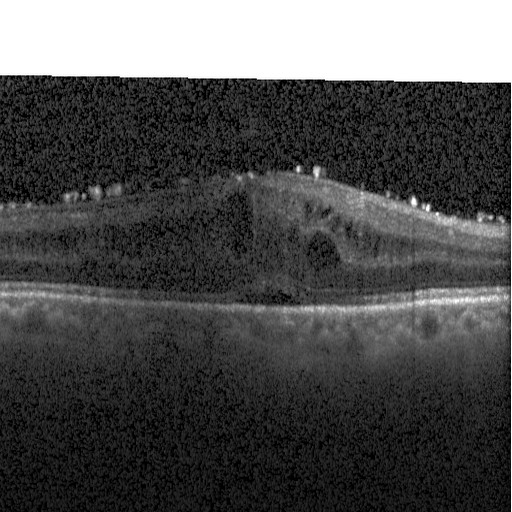
Through the macula. Retinal OCT B-scan. SD-OCT. Heidelberg Spectralis. Finding: diabetic macular edema (DME).